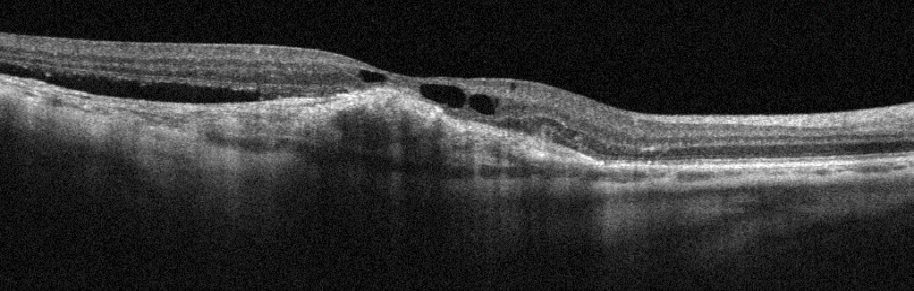
OCT B-scan · oculus dexter.
Diagnosis: age-related macular degeneration.